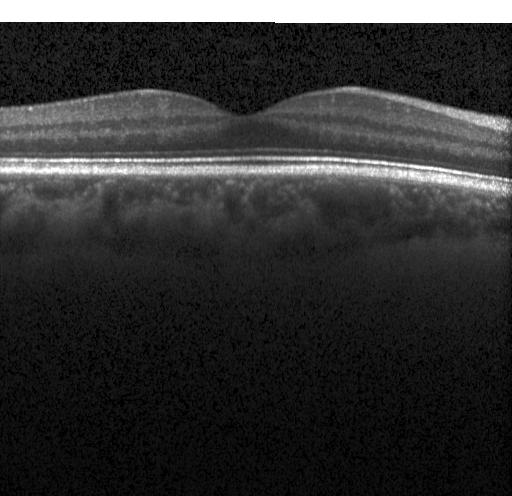 Impression: no choroidal neovascularization, no diabetic macular edema, and no drusen.